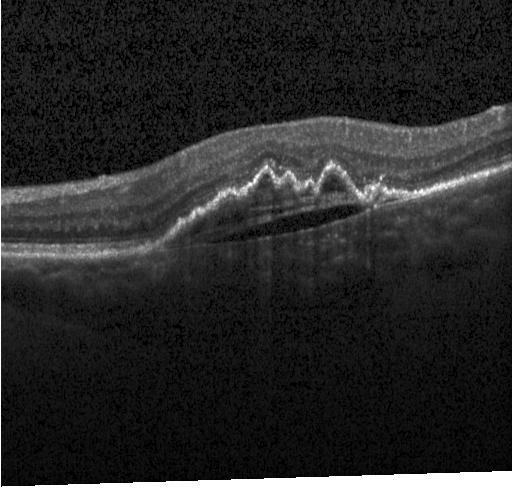

Macular OCT: CNV.